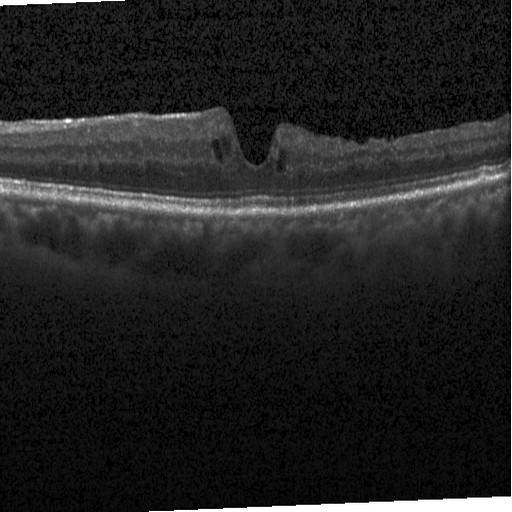
Diagnosis: diabetic macular edema (DME).